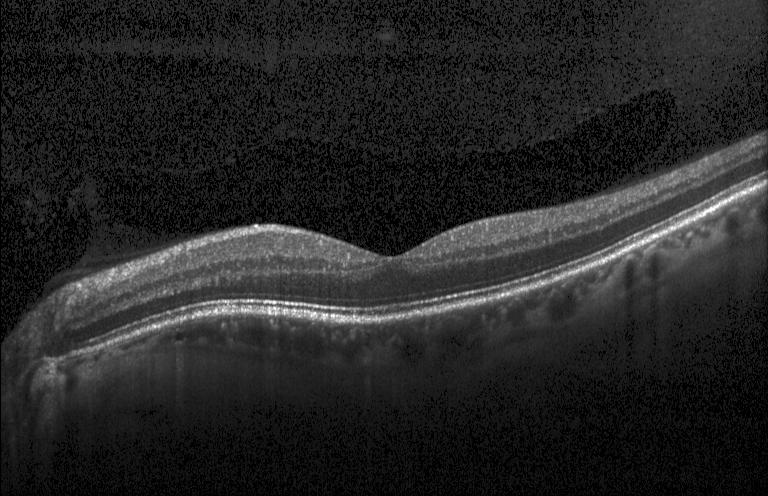

Finding: neither choroidal neovascularization, diabetic macular edema, nor drusen.